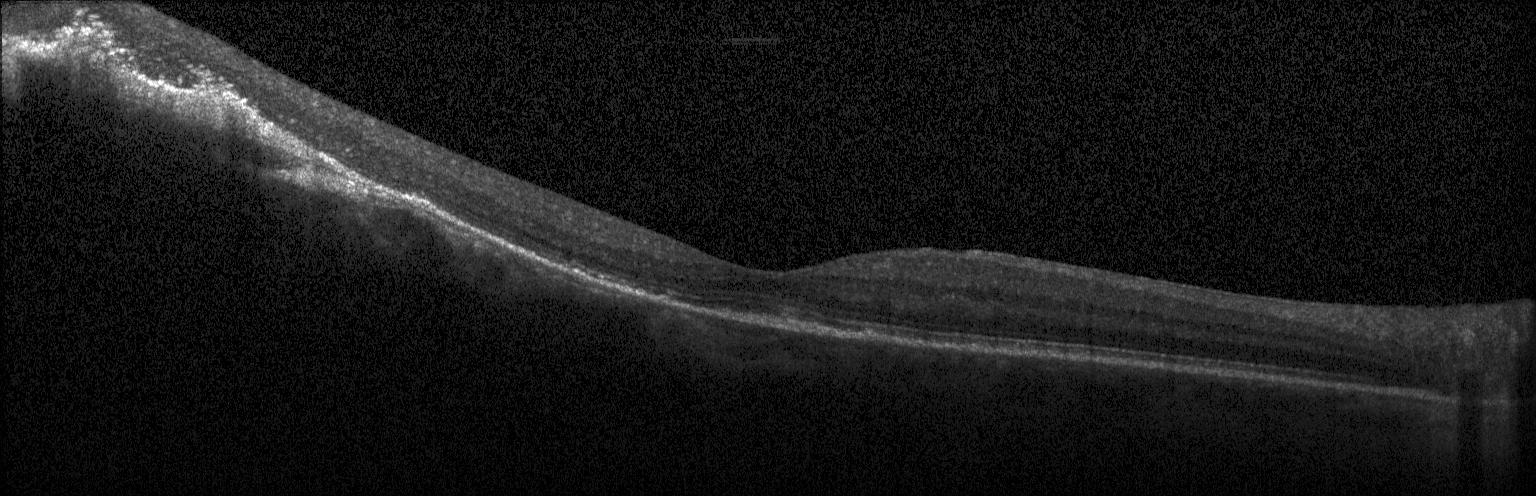

Diagnosis: a choroidal neovascular membrane.